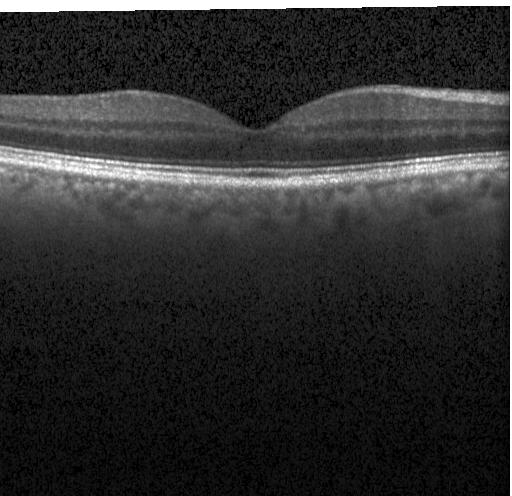 Diagnosis: no CNV, no DME, and no drusen.